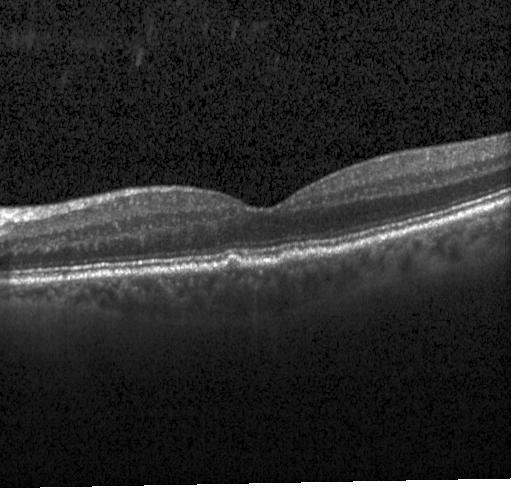
Spectral-domain optical coherence tomography. Optical coherence tomography scan — OCT finding: multiple drusen.